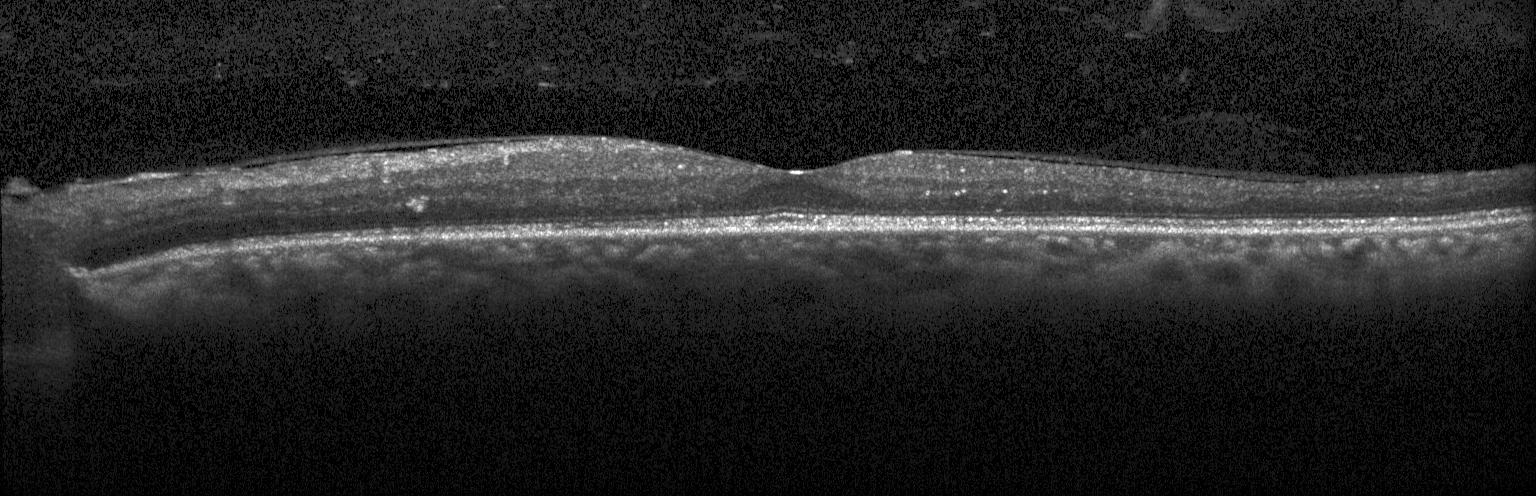 Retinal OCT B-scan — Diagnosis: diabetic macular edema (DME).